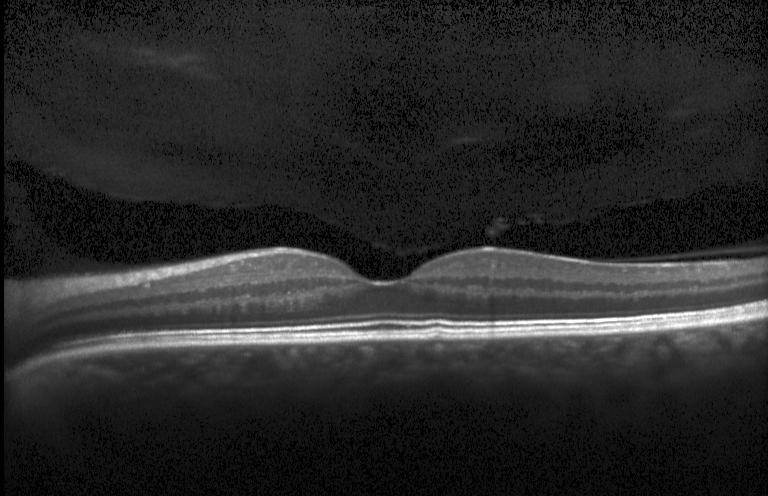

Instrument: Heidelberg Spectralis, OCT B-scan, centered on the fovea — Impression: no CNV, DME, or drusen.